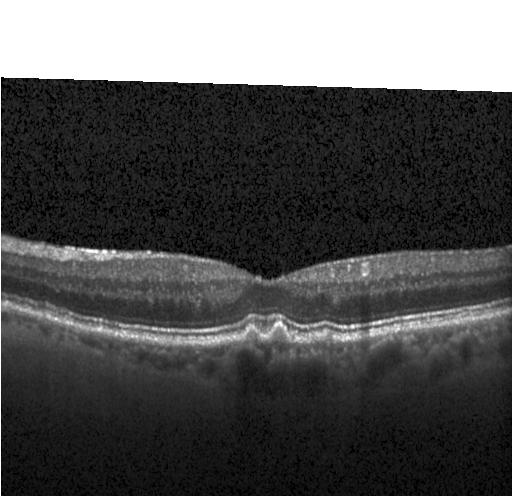

SD-OCT, retinal OCT B-scan
Drusen.